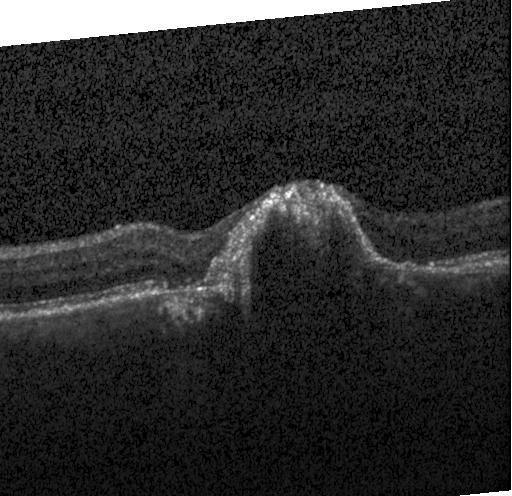

Acquired on a Heidelberg Spectralis, optical coherence tomography scan — Diagnosis: CNV.